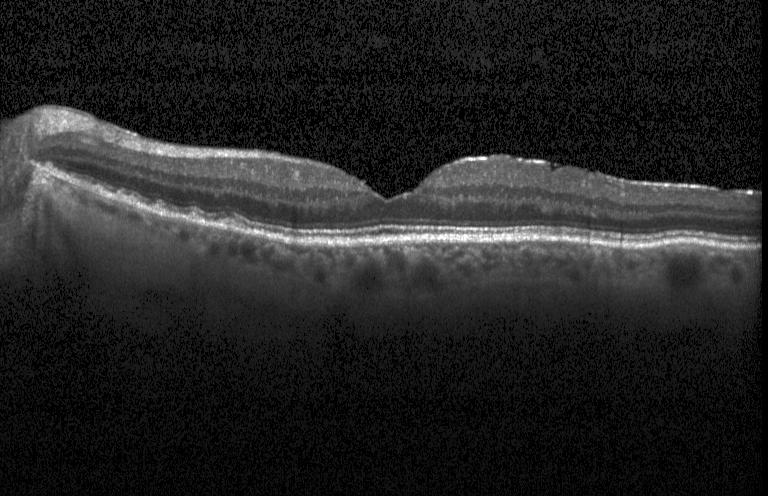 Retinal OCT B-scan
This B-scan demonstrates sub-RPE drusenoid deposits.